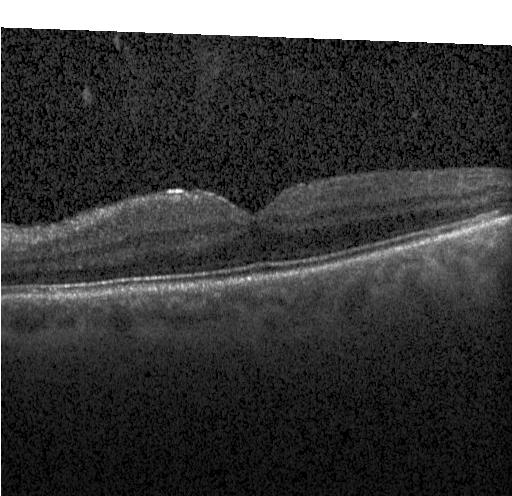 Retinal OCT B-scan, horizontal scan through the fovea
Neither choroidal neovascularization, diabetic macular edema, nor drusen.